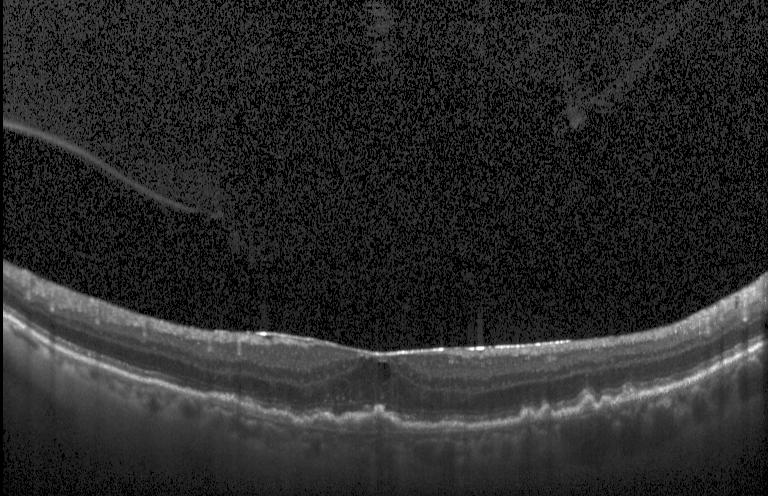 SD-OCT · Heidelberg Spectralis · OCT line scan · centered on the fovea.
Impression: choroidal neovascularization.